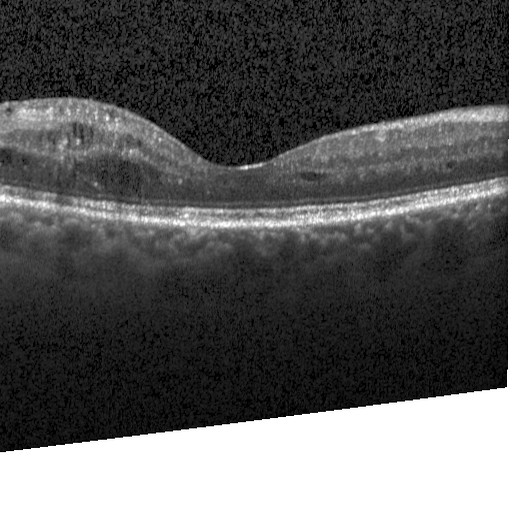
Finding: diabetic macular edema (DME).